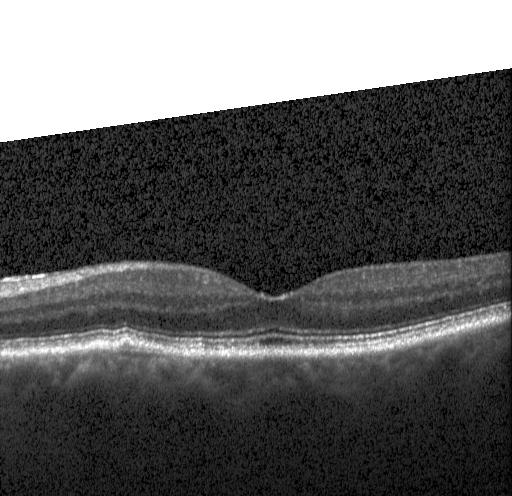

Acquired on a Heidelberg Spectralis. OCT B-scan. Spectral-domain optical coherence tomography. Horizontal scan through the fovea
Dx: multiple drusen.